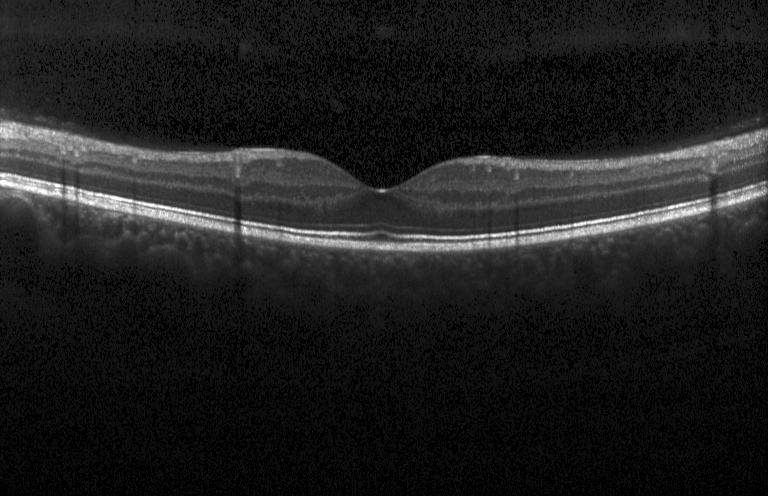 Diagnosis: neither CNV, DME, nor drusen.